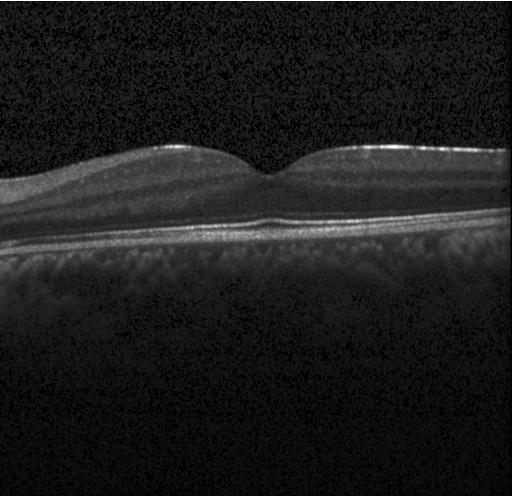
Heidelberg Spectralis. Retinal OCT cross-section. Spectral-domain OCT. Fovea-centered
Finding: no choroidal neovascularization, diabetic macular edema, or drusen.